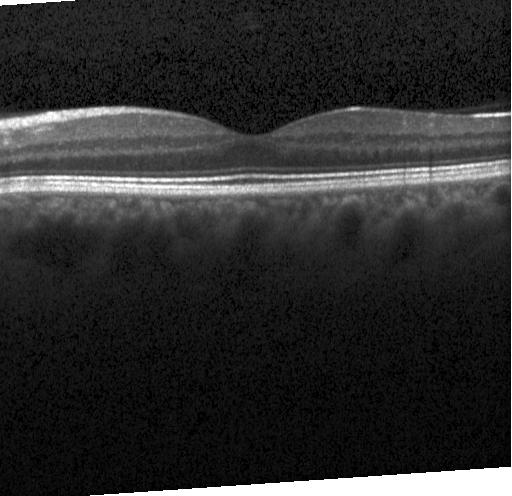
OCT line scan
Diagnosis: neither choroidal neovascularization, diabetic macular edema, nor drusen.